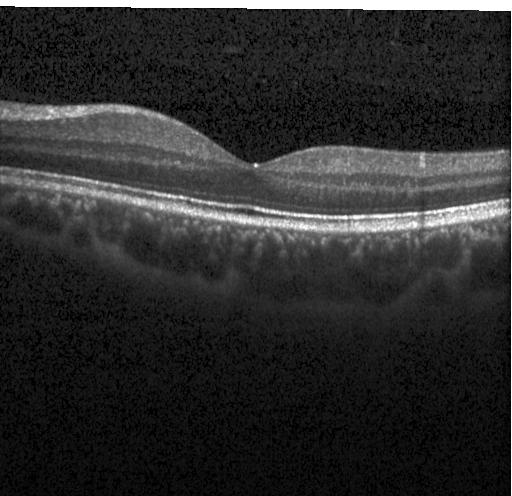

Diagnosis: no evidence of choroidal neovascularization, diabetic macular edema, or drusen.